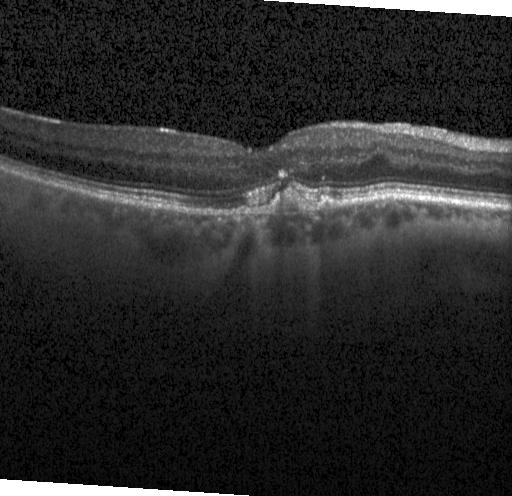 Finding: CNV.